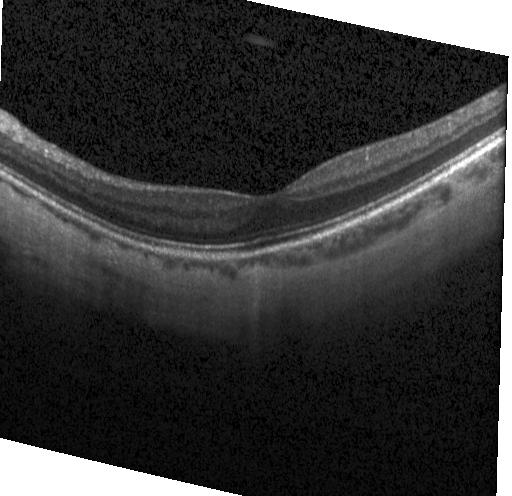
Retinal OCT cross-section.
Impression: no evidence of choroidal neovascularization, diabetic macular edema, or drusen.